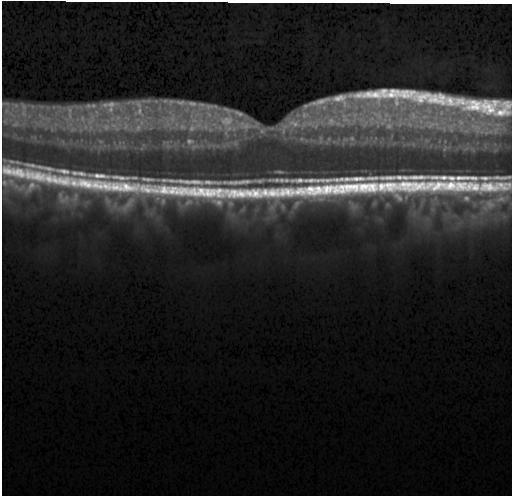

Horizontal scan through the fovea · optical coherence tomography B-scan · acquired on a Heidelberg Spectralis
No choroidal neovascularization, no diabetic macular edema, and no drusen.